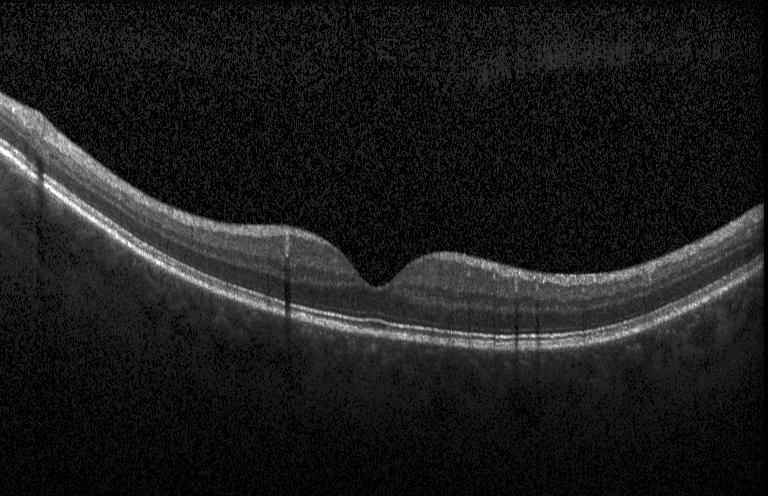

Diagnosis: neither CNV, DME, nor drusen.